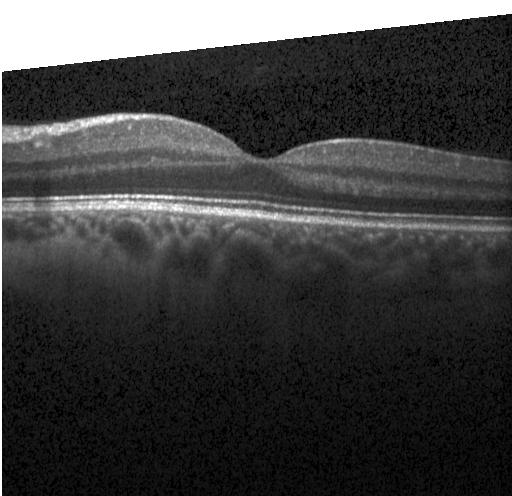

OCT finding: no evidence of choroidal neovascularization, diabetic macular edema, or drusen.